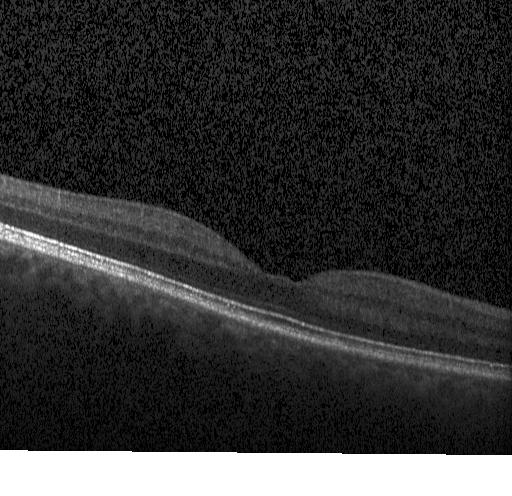
Retinal OCT B-scan. No CNV, no DME, and no drusen.